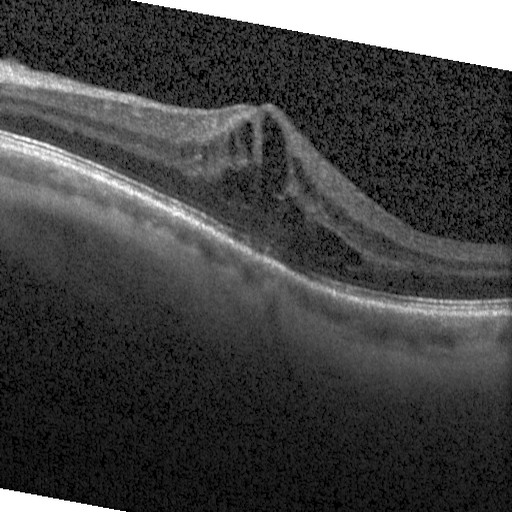

OCT scan showing diabetic macular edema.